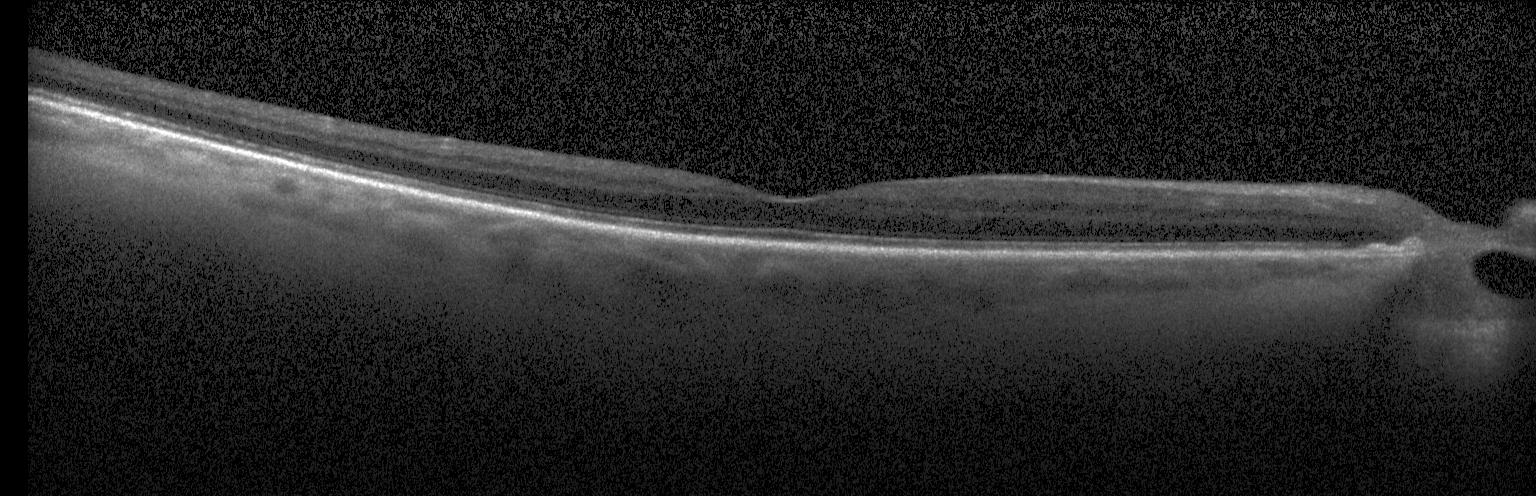
Macular OCT: no CNV, DME, or drusen.